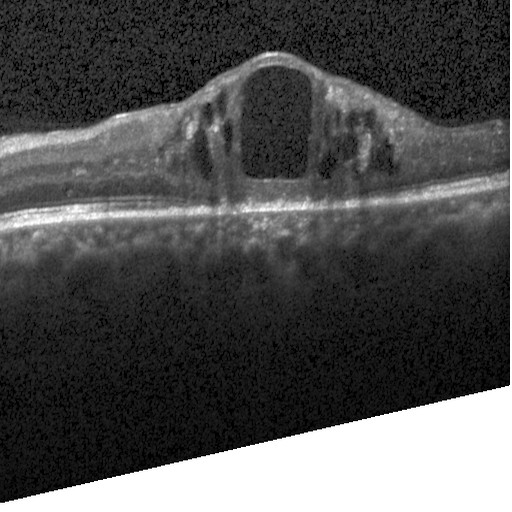
Acquired on a Heidelberg Spectralis; retinal OCT B-scan — Diagnosis: DME.